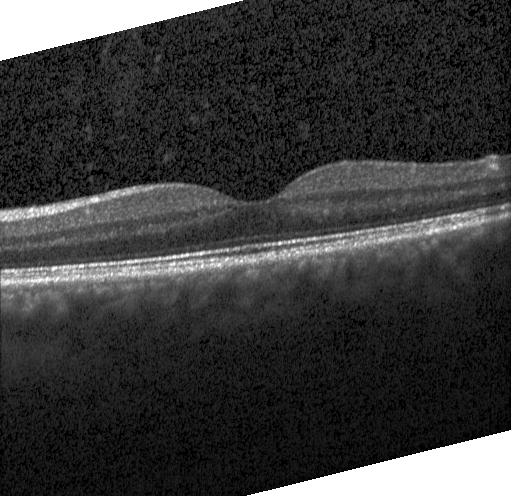

OCT scan showing no choroidal neovascularization, no diabetic macular edema, and no drusen.